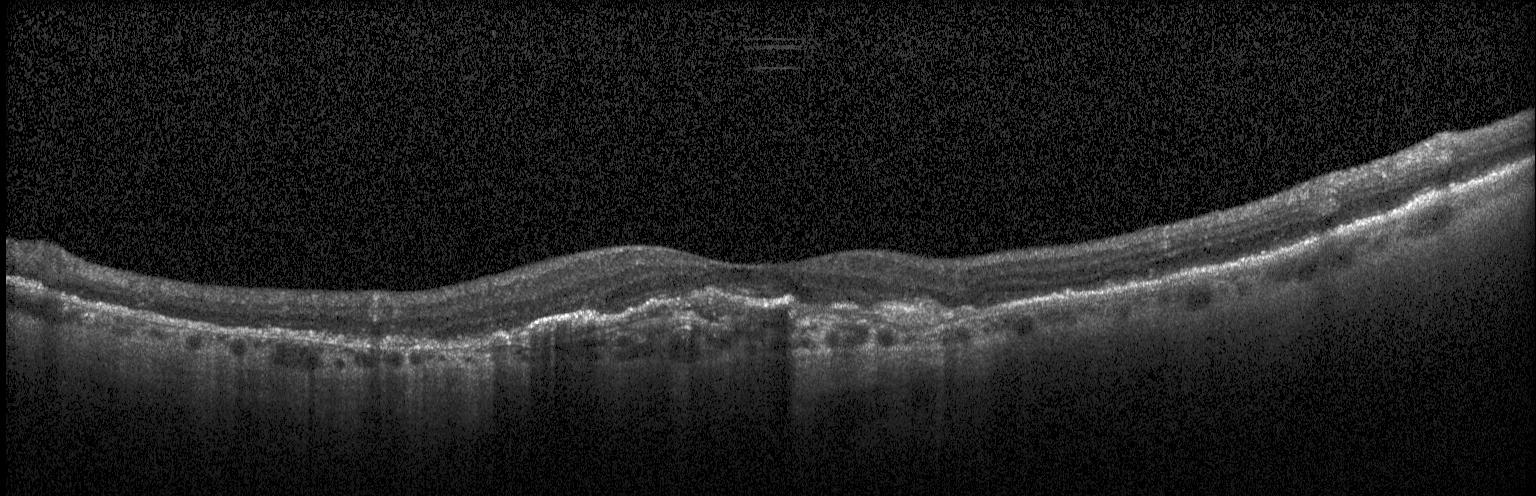

Spectral-domain OCT B-scan: choroidal neovascularization.